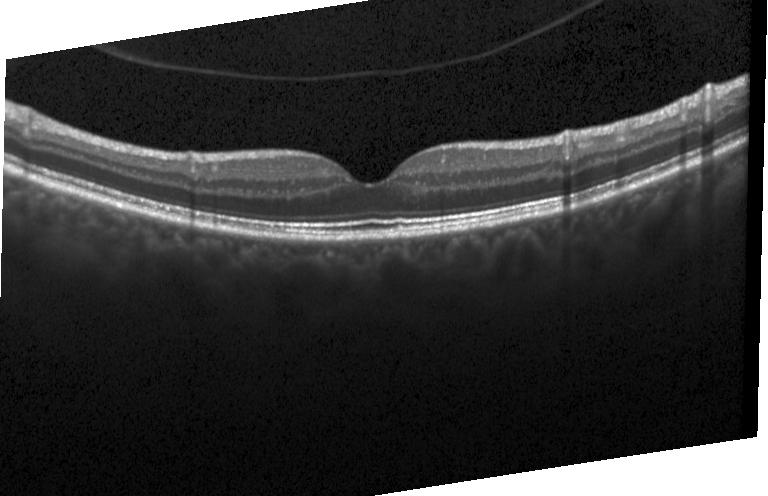

Through the macula. Optical coherence tomography scan. Acquired on a Heidelberg Spectralis. Spectral-domain OCT
This B-scan demonstrates no CNV, DME, or drusen.